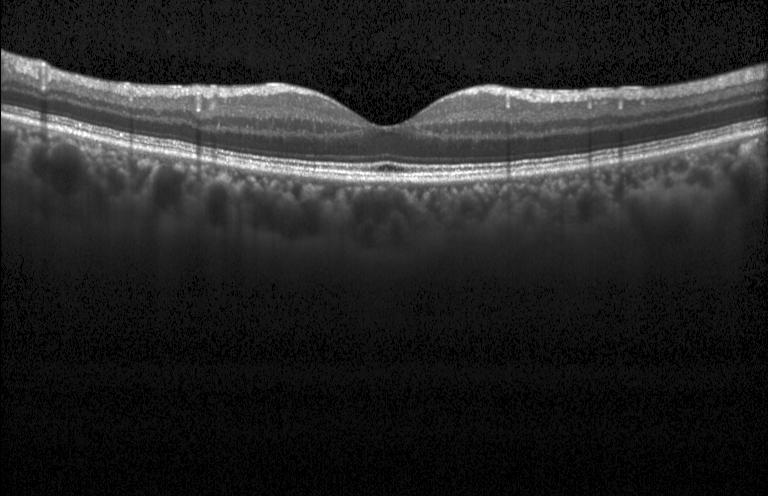 This B-scan demonstrates no choroidal neovascularization, no diabetic macular edema, and no drusen.